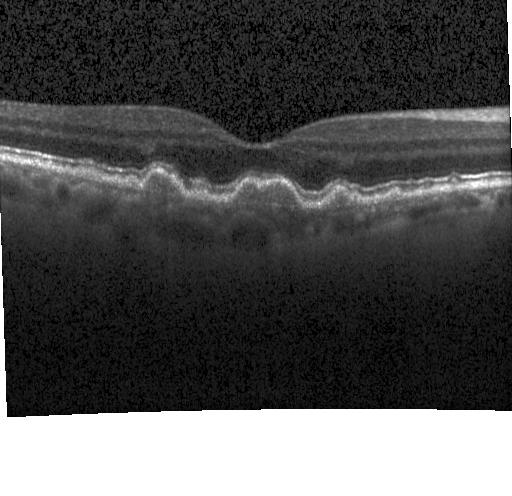
Optical coherence tomography scan.
Finding: drusen.